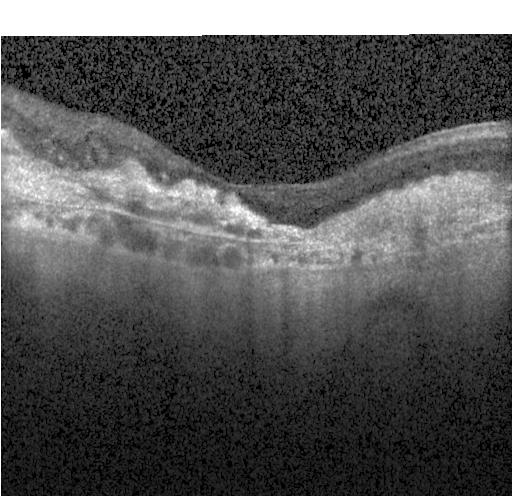
SD-OCT · optical coherence tomography scan. Finding: choroidal neovascularization.